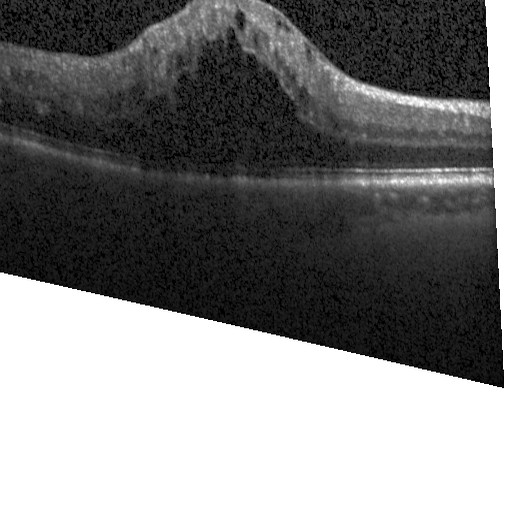 Macular scan · Heidelberg Spectralis · OCT line scan
Finding: DME.